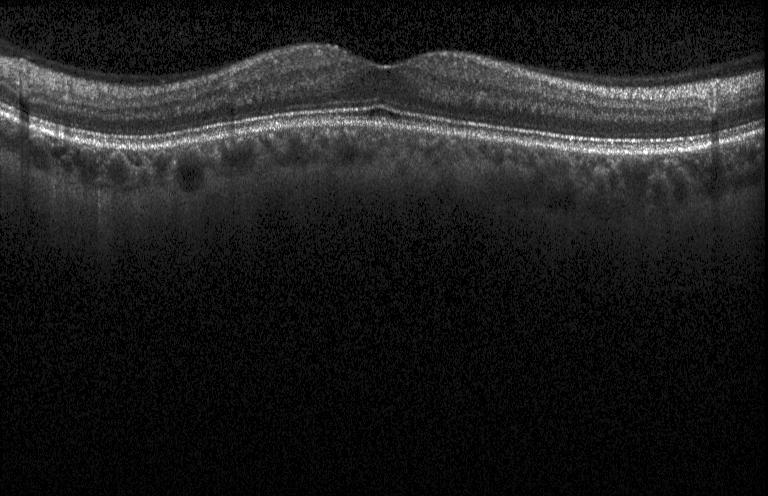

No choroidal neovascularization, diabetic macular edema, or drusen.